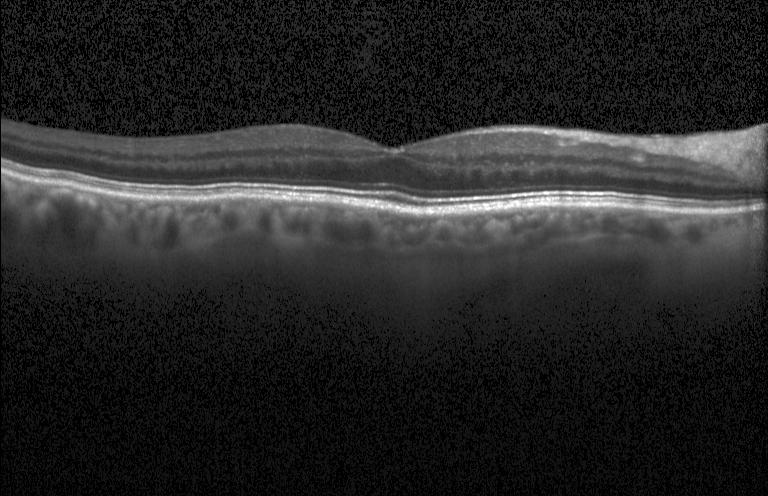 Heidelberg Spectralis OCT system · optical coherence tomography B-scan
Impression: no choroidal neovascularization, no diabetic macular edema, and no drusen.